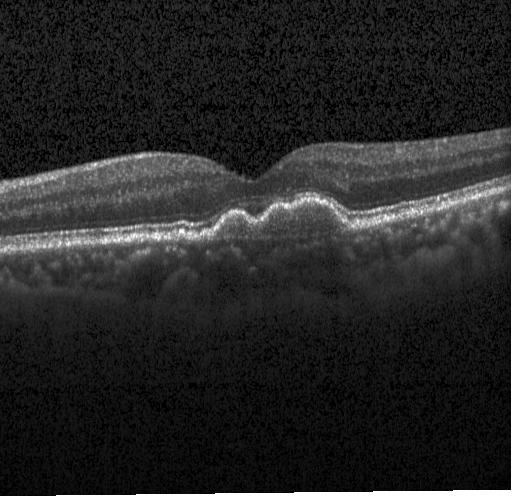

Multiple drusen.